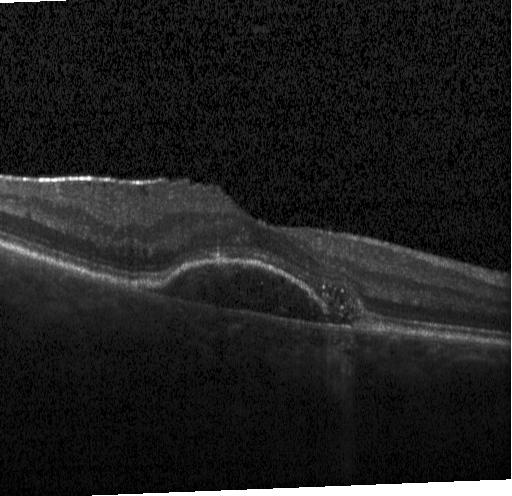

This B-scan demonstrates choroidal neovascularization.